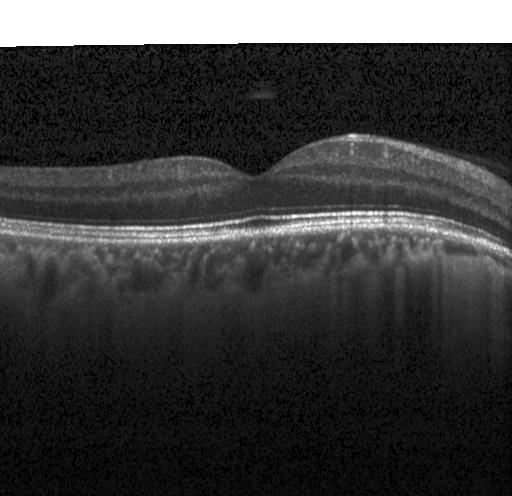 OCT line scan — This B-scan demonstrates no evidence of choroidal neovascularization, diabetic macular edema, or drusen.